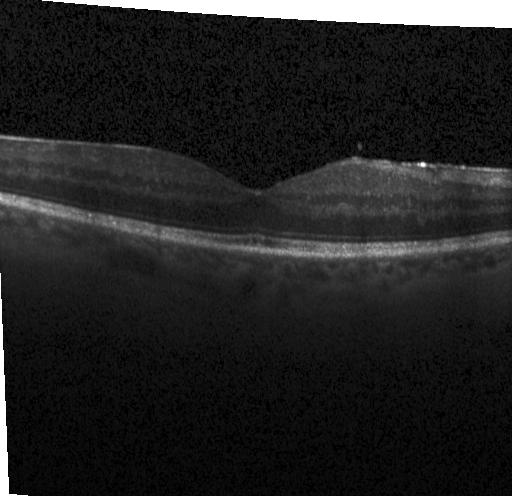

Impression: no evidence of choroidal neovascularization, diabetic macular edema, or drusen.